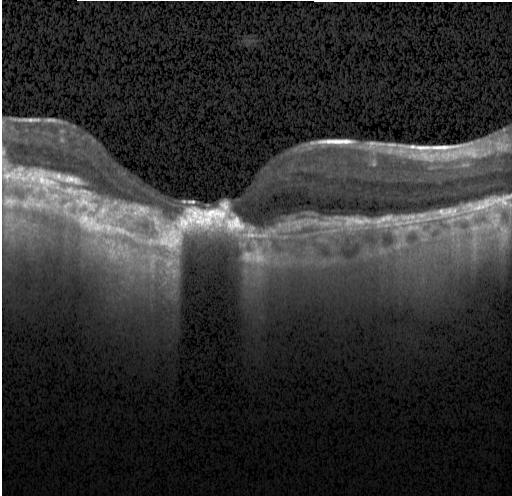

Assessment: choroidal neovascularization (CNV).